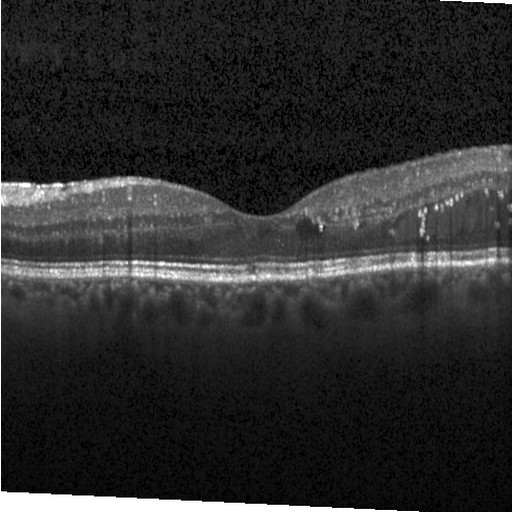
Diagnosis: DME.